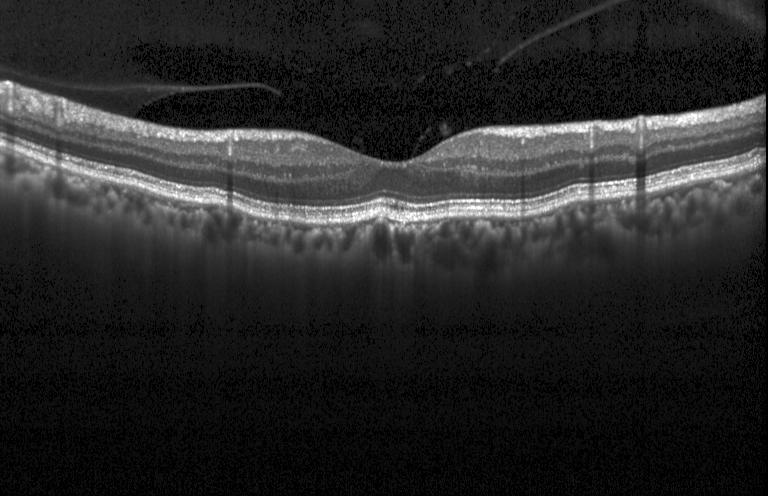

Retinal OCT cross-section
Finding: multiple drusen.